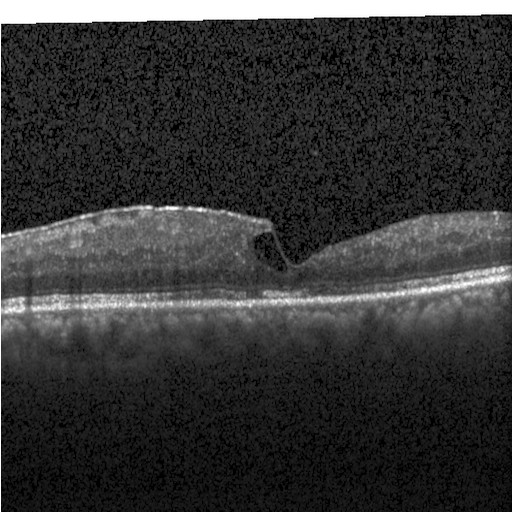 Fovea-centered. Optical coherence tomography scan. Instrument: Heidelberg Spectralis — Assessment: diabetic macular edema (DME).